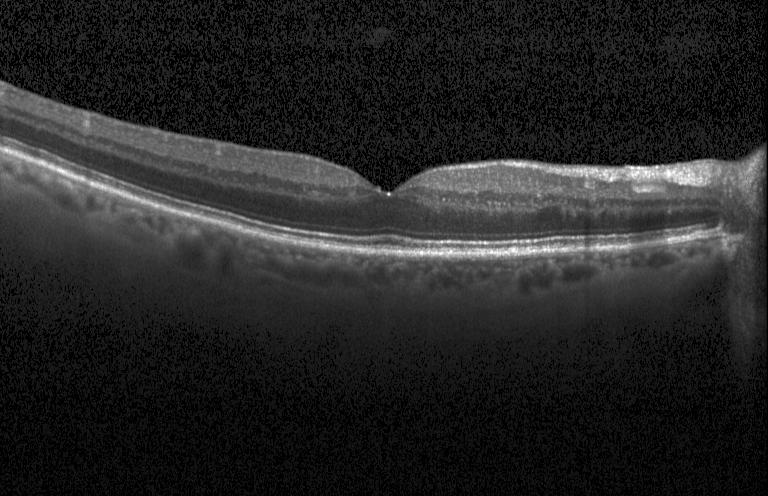
Through the macula. Spectral-domain optical coherence tomography. Retinal OCT B-scan — Diagnosis: no choroidal neovascularization, no diabetic macular edema, and no drusen.